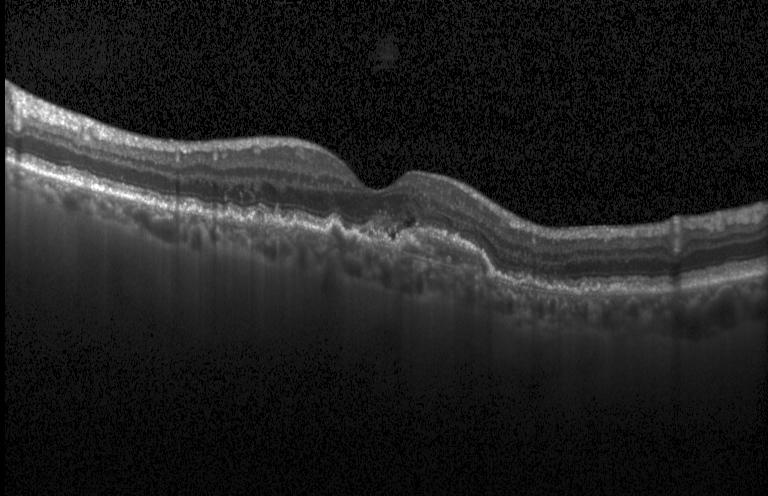 Diagnosis: a choroidal neovascular membrane.